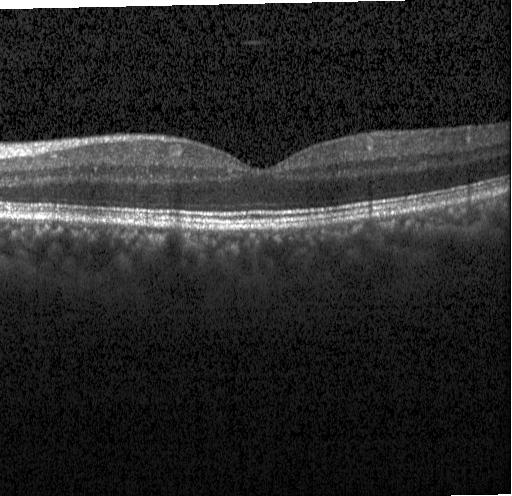

Retinal OCT B-scan. No choroidal neovascularization, no diabetic macular edema, and no drusen.